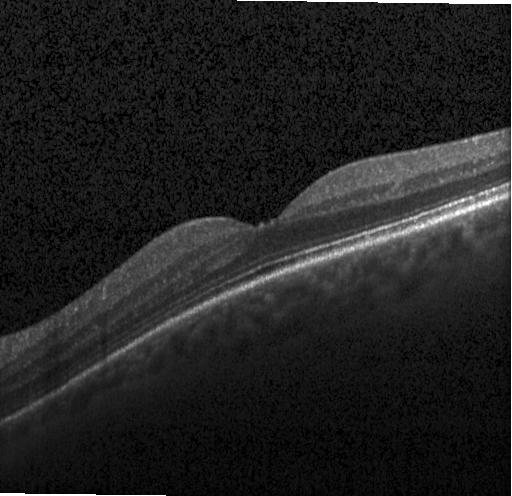 OCT finding: no evidence of choroidal neovascularization, diabetic macular edema, or drusen.